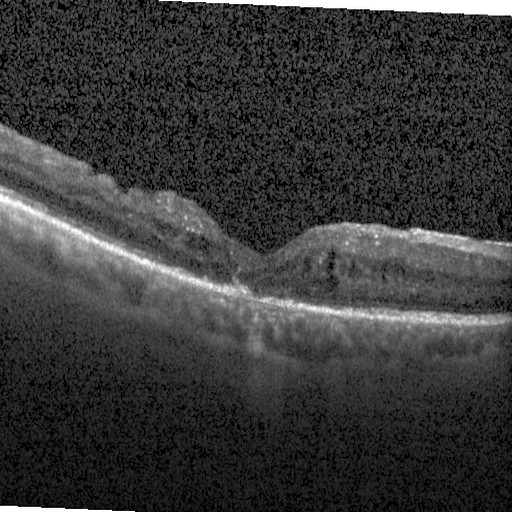

OCT line scan — Diagnosis: diabetic macular edema (DME).